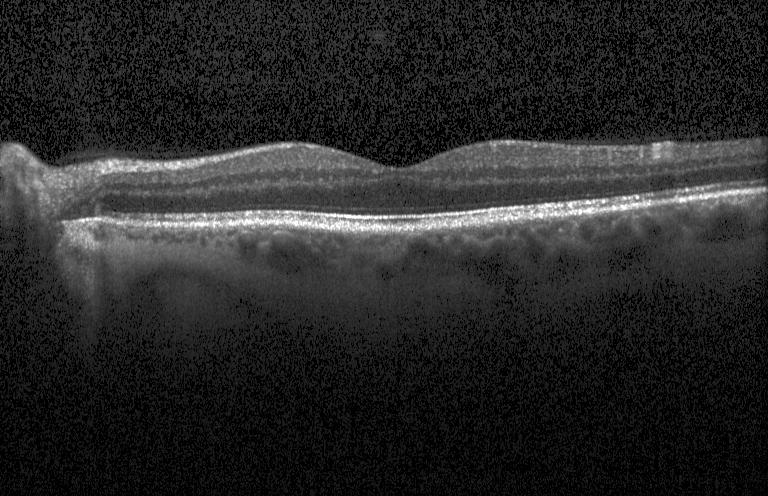 OCT scan showing no choroidal neovascularization, diabetic macular edema, or drusen.